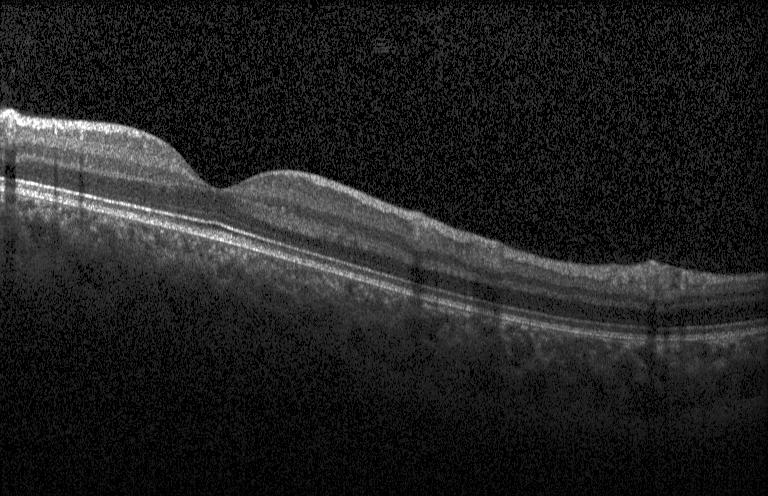
SD-OCT; retinal OCT B-scan; Heidelberg Spectralis OCT system — Diagnosis: no choroidal neovascularization, diabetic macular edema, or drusen.